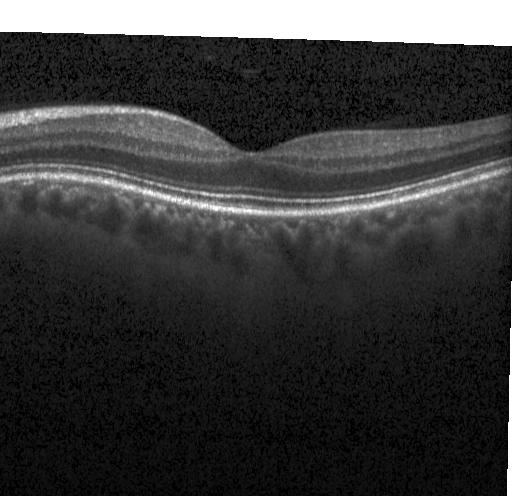
Optical coherence tomography scan
Dx: no CNV, DME, or drusen.